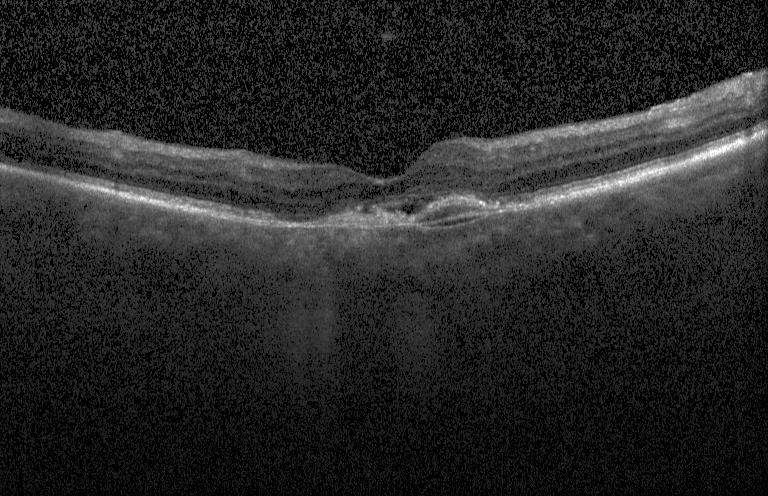
This B-scan demonstrates CNV.